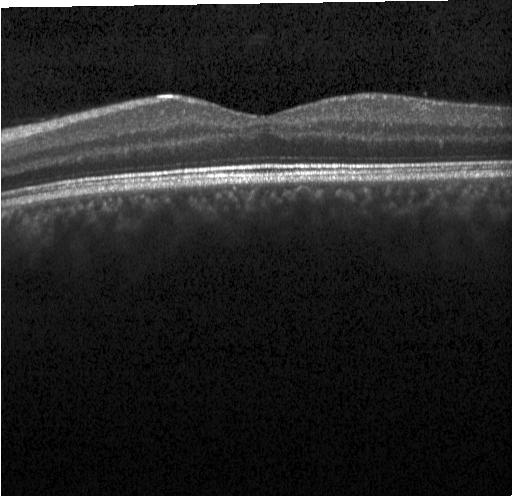

Dx: no evidence of choroidal neovascularization, diabetic macular edema, or drusen.